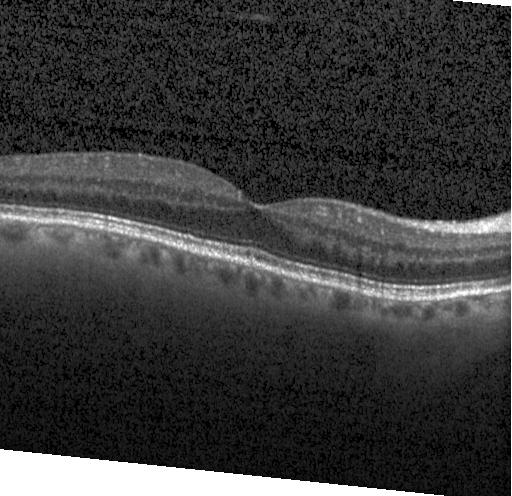
Heidelberg Spectralis OCT system, optical coherence tomography B-scan.
The scan shows neither choroidal neovascularization, diabetic macular edema, nor drusen.